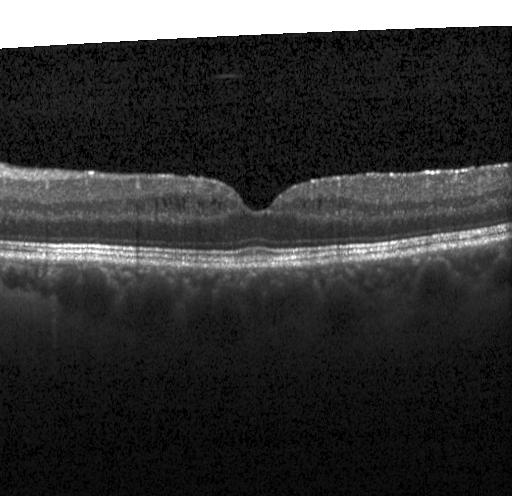 Optical coherence tomography B-scan; spectral-domain optical coherence tomography; Heidelberg Spectralis; through the macula
Finding: DME.